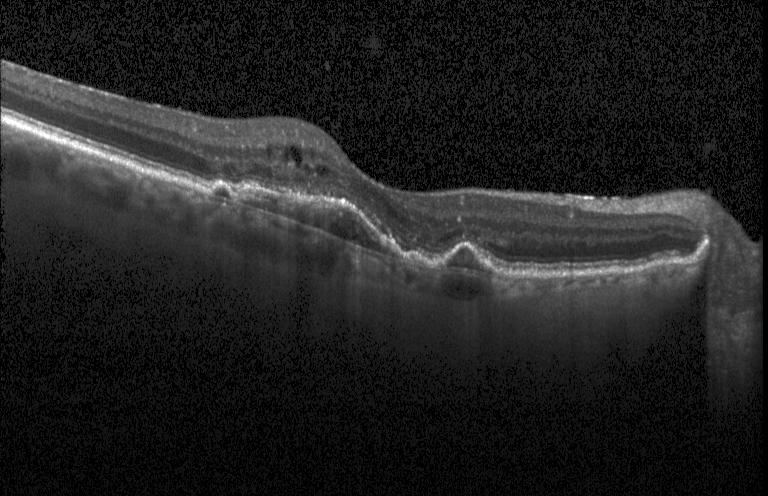

OCT finding: a choroidal neovascular membrane.